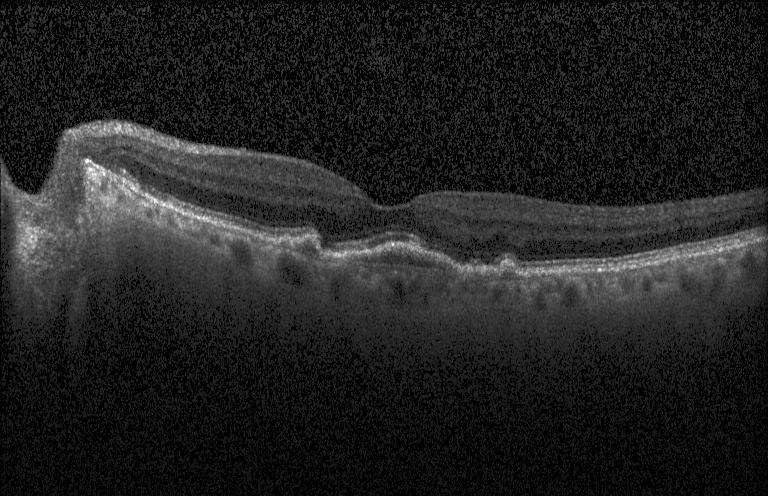
Retinal OCT B-scan.
A choroidal neovascular membrane.